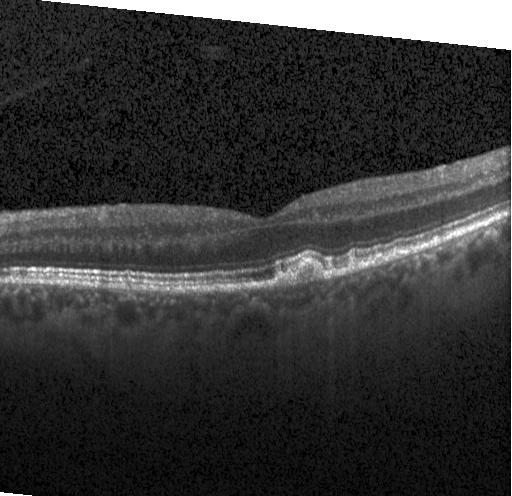
OCT B-scan · macular scan — Finding: sub-RPE drusenoid deposits.